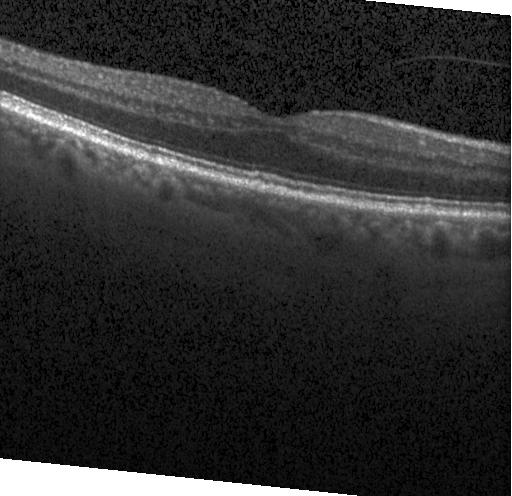 Diagnosis: no choroidal neovascularization, diabetic macular edema, or drusen.